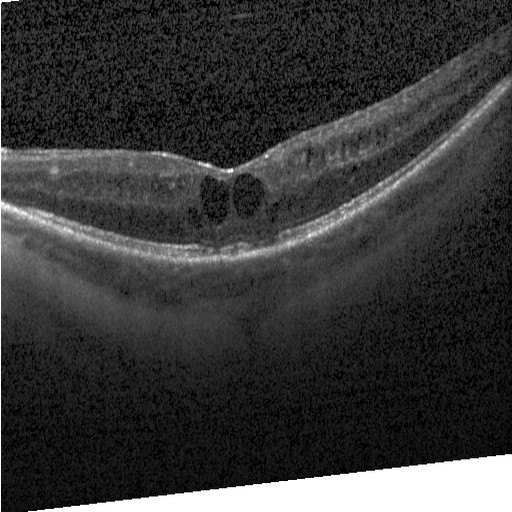
Macular OCT: diabetic macular edema (DME).